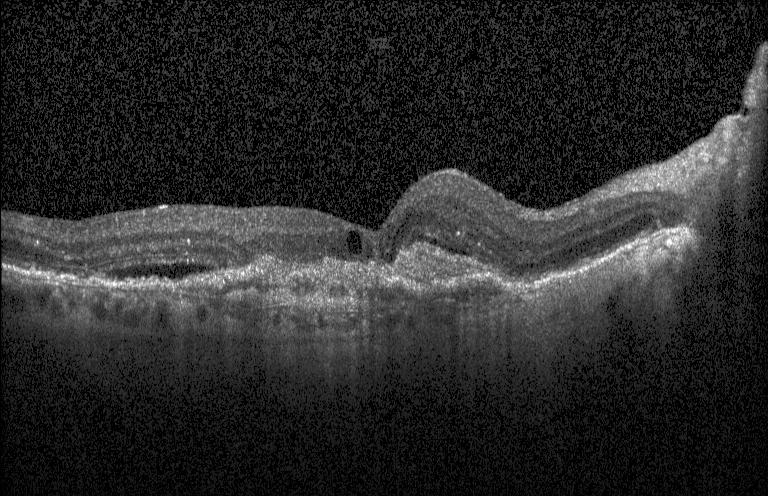

Spectral-domain optical coherence tomography. Macular scan. Optical coherence tomography B-scan. Heidelberg Spectralis — Impression: a choroidal neovascular membrane.